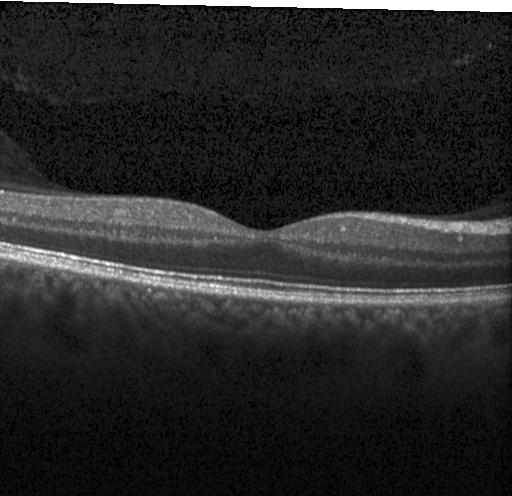
Spectral-domain optical coherence tomography, Heidelberg Spectralis, optical coherence tomography scan, horizontal scan through the fovea.
Finding: no evidence of CNV, DME, or drusen.